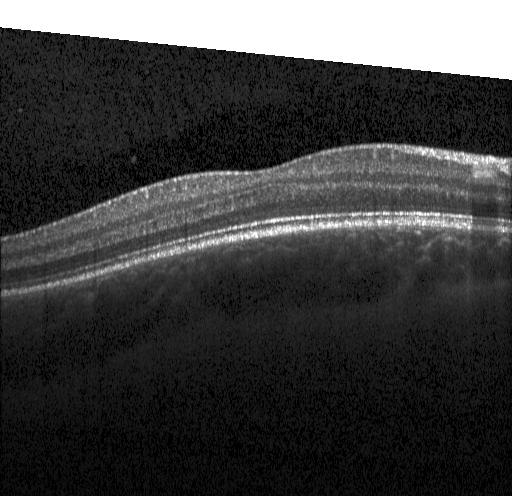

SD-OCT; instrument: Heidelberg Spectralis; optical coherence tomography B-scan; through the macula — Finding: no CNV, no DME, and no drusen.